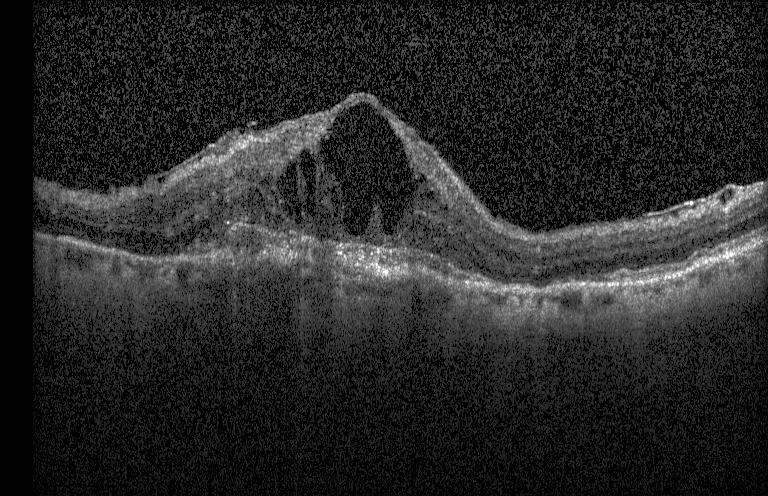
Optical coherence tomography B-scan
Finding: choroidal neovascularization (CNV).